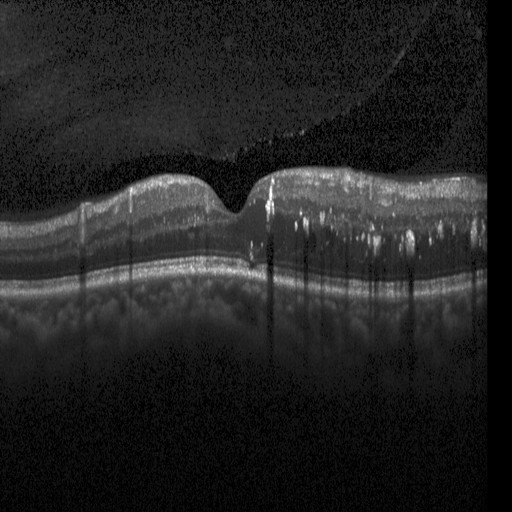

Retinal OCT B-scan. Finding: DME.